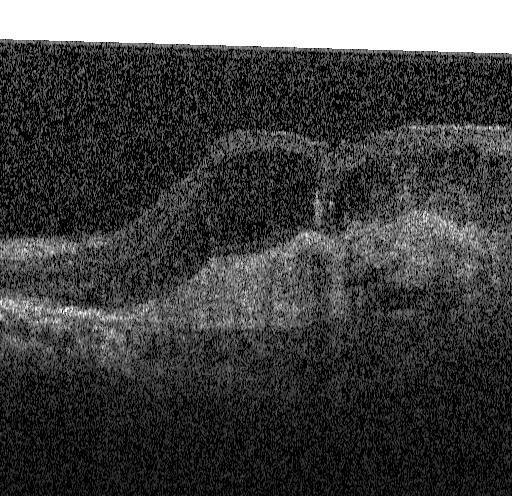 Heidelberg Spectralis OCT system · spectral-domain optical coherence tomography · optical coherence tomography B-scan · through the macula — Impression: choroidal neovascularization.